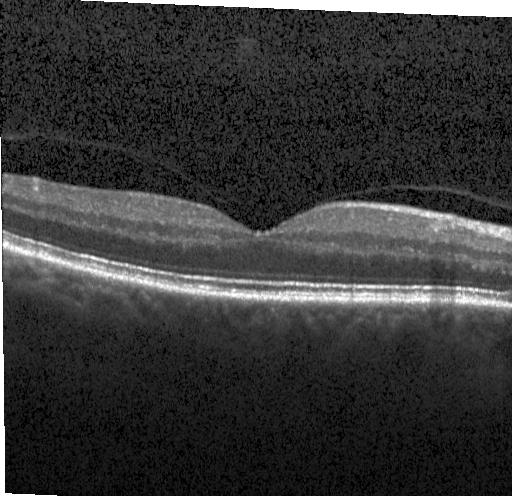

Optical coherence tomography scan; spectral-domain OCT
Diagnosis: no choroidal neovascularization, no diabetic macular edema, and no drusen.